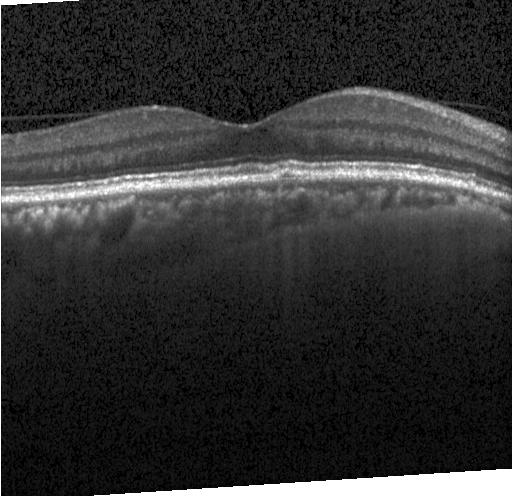
Impression: multiple drusen.